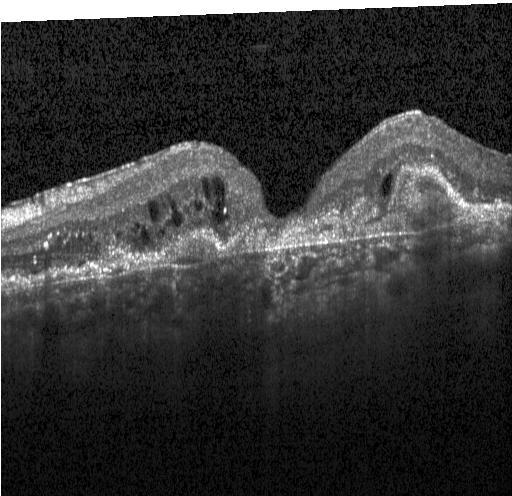

OCT B-scan, spectral-domain optical coherence tomography, centered on the fovea. This B-scan demonstrates choroidal neovascularization (CNV).